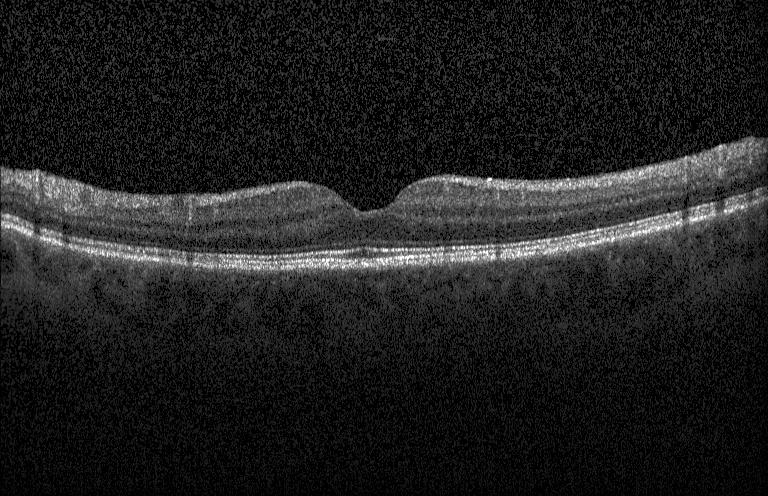 Spectral-domain OCT · Heidelberg Spectralis OCT system · retinal OCT cross-section.
Diagnosis: neither CNV, DME, nor drusen.